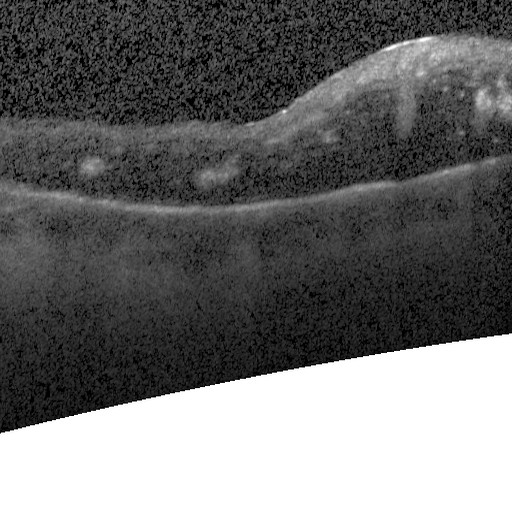

Heidelberg Spectralis. SD-OCT. OCT B-scan. Fovea-centered. Diagnosis: diabetic macular edema (DME).